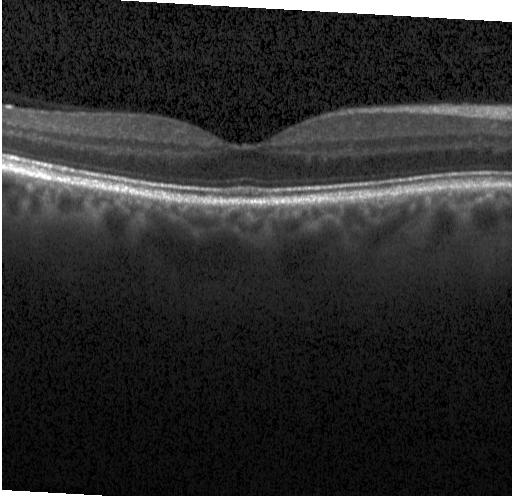 Acquired on a Heidelberg Spectralis. SD-OCT. OCT line scan — No CNV, no DME, and no drusen.